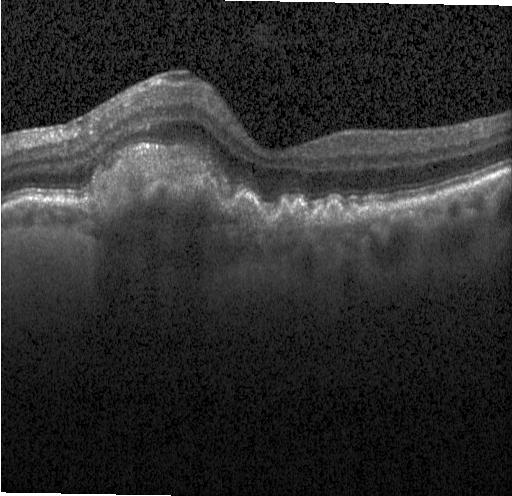 Macular OCT: CNV.